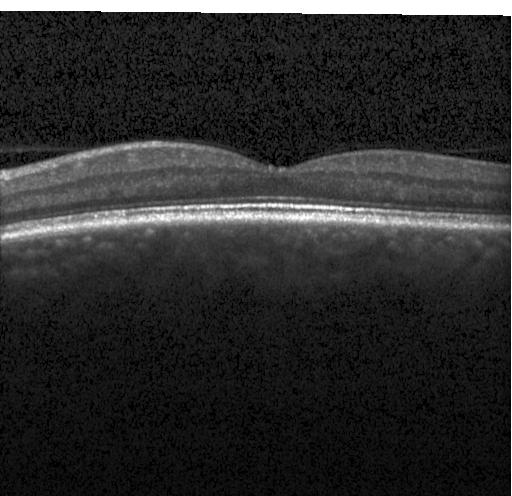 Optical coherence tomography scan — Impression: no choroidal neovascularization, diabetic macular edema, or drusen.